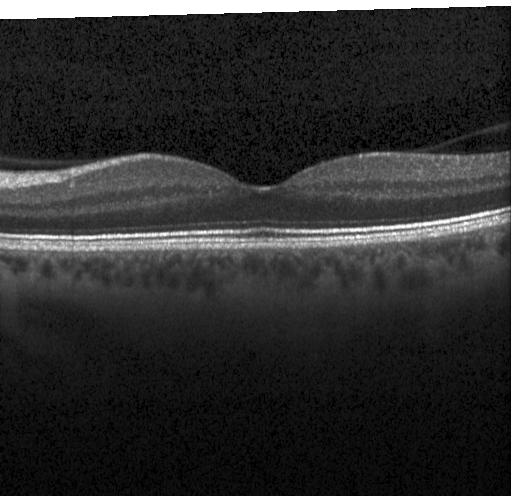
Retinal OCT B-scan; centered on the fovea — Diagnosis: no evidence of CNV, DME, or drusen.